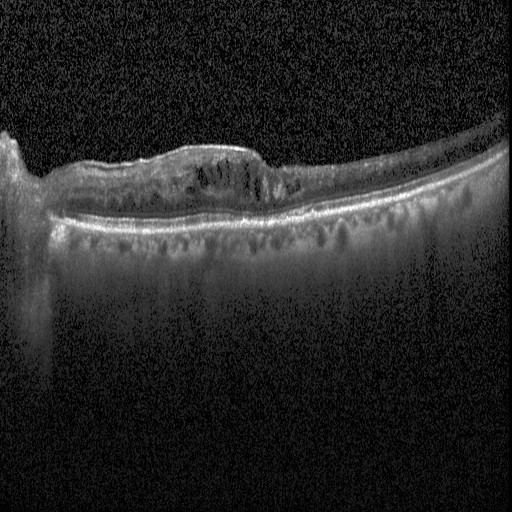

OCT B-scan. Heidelberg Spectralis. Macular scan. SD-OCT.
Dx: diabetic macular edema (DME).